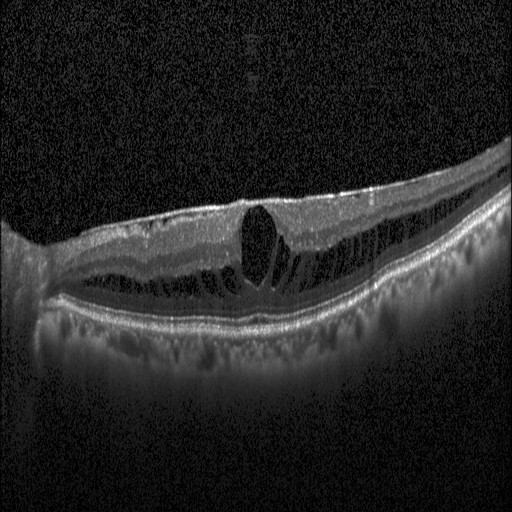 OCT line scan.
The scan shows diabetic macular edema (DME).